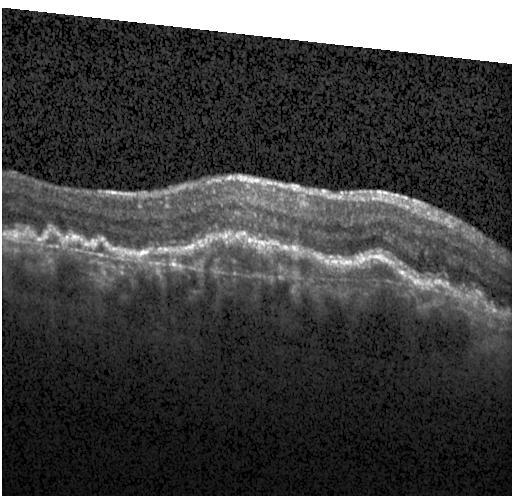 Through the macula · Heidelberg Spectralis · retinal OCT B-scan · spectral-domain OCT.
Diagnosis: choroidal neovascularization (CNV).